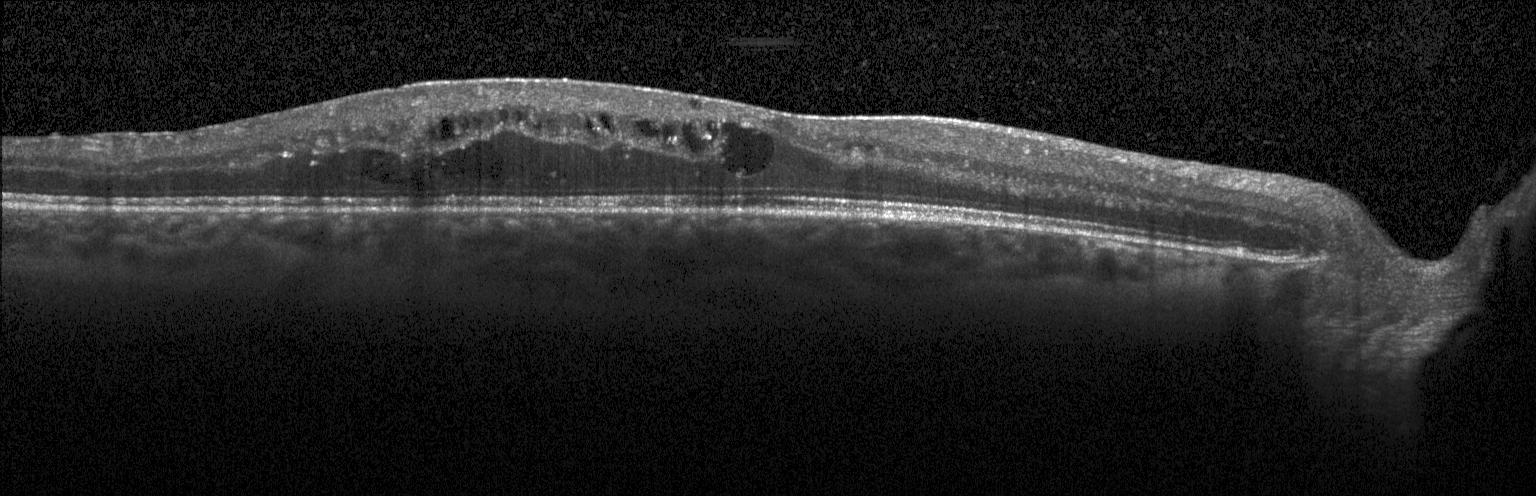

Impression: diabetic macular edema.